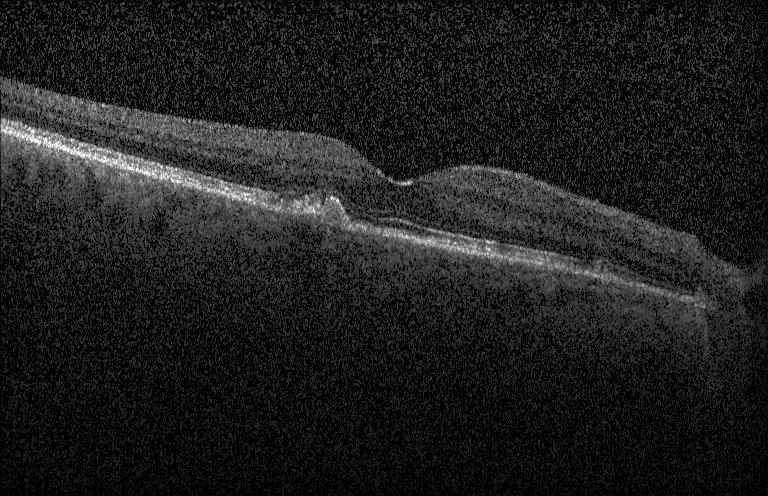
Choroidal neovascularization.